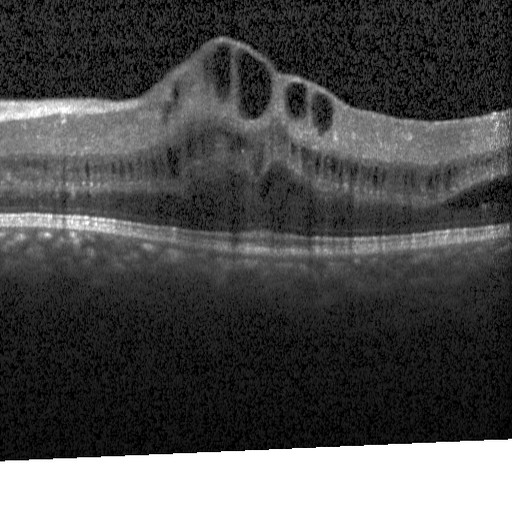
Macular OCT demonstrating diabetic macular edema (DME).